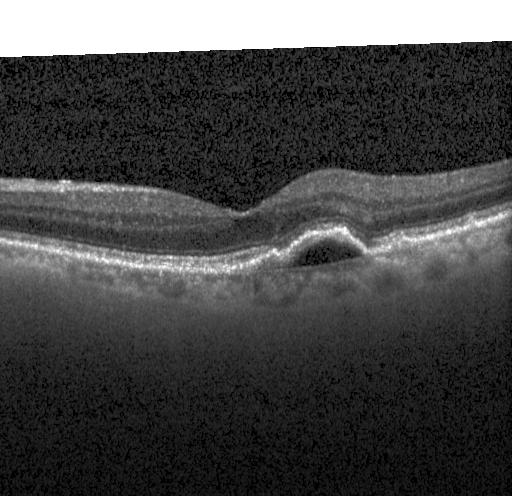 Retinal OCT B-scan. Spectral-domain OCT.
CNV.